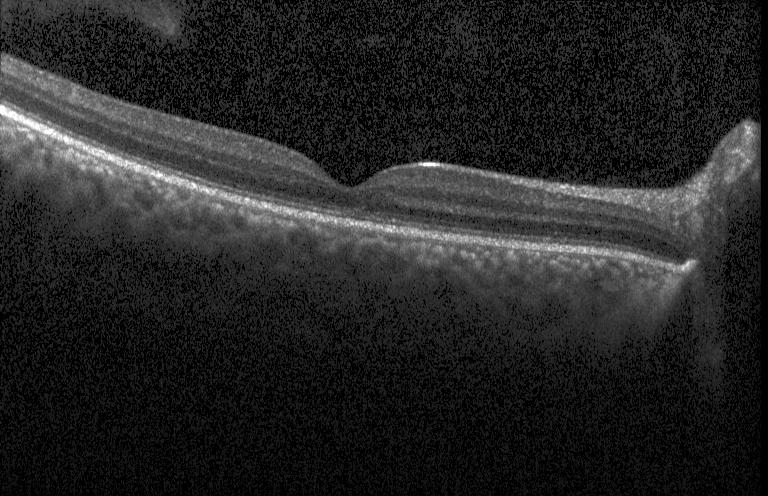

SD-OCT; macular scan; instrument: Heidelberg Spectralis; retinal OCT B-scan
No choroidal neovascularization, diabetic macular edema, or drusen.